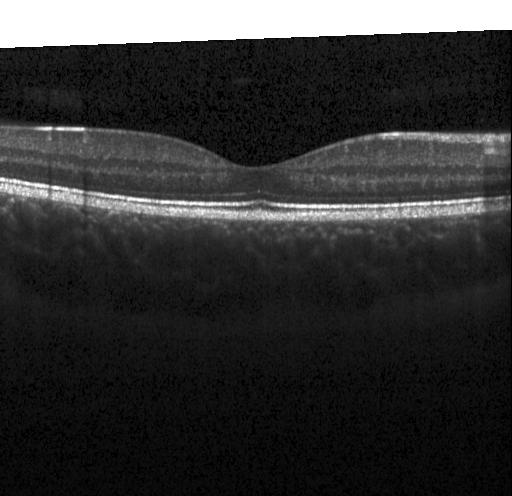
Dx: no choroidal neovascularization, no diabetic macular edema, and no drusen.